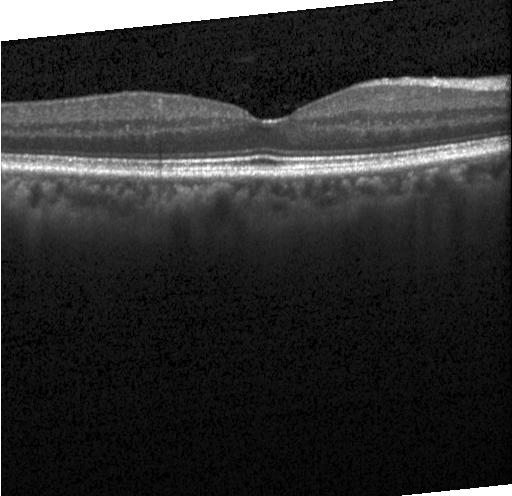 This B-scan demonstrates no choroidal neovascularization, no diabetic macular edema, and no drusen.